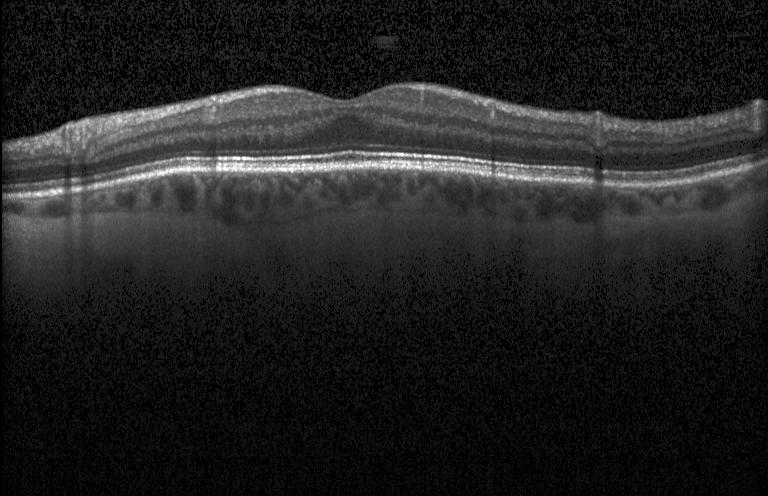

Optical coherence tomography B-scan.
Impression: no evidence of choroidal neovascularization, diabetic macular edema, or drusen.